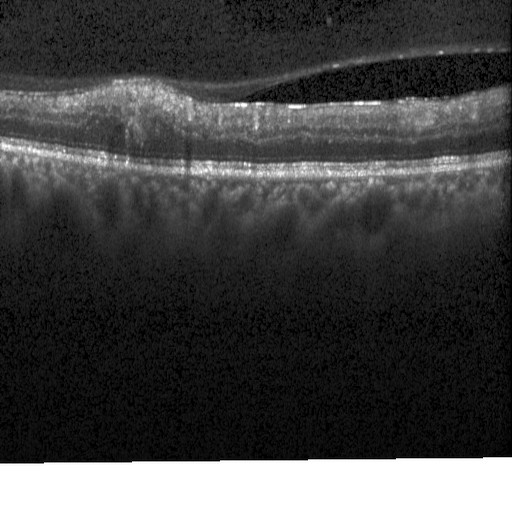 Spectral-domain OCT, optical coherence tomography scan.
Finding: diabetic macular edema (DME).